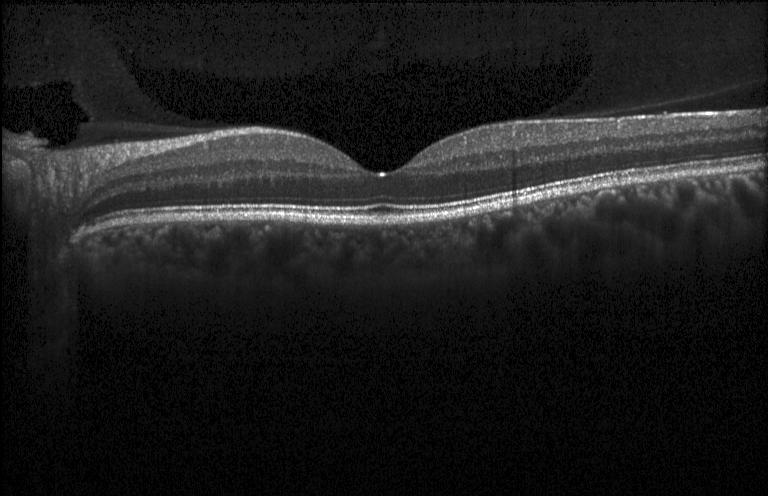
Dx: no evidence of choroidal neovascularization, diabetic macular edema, or drusen.